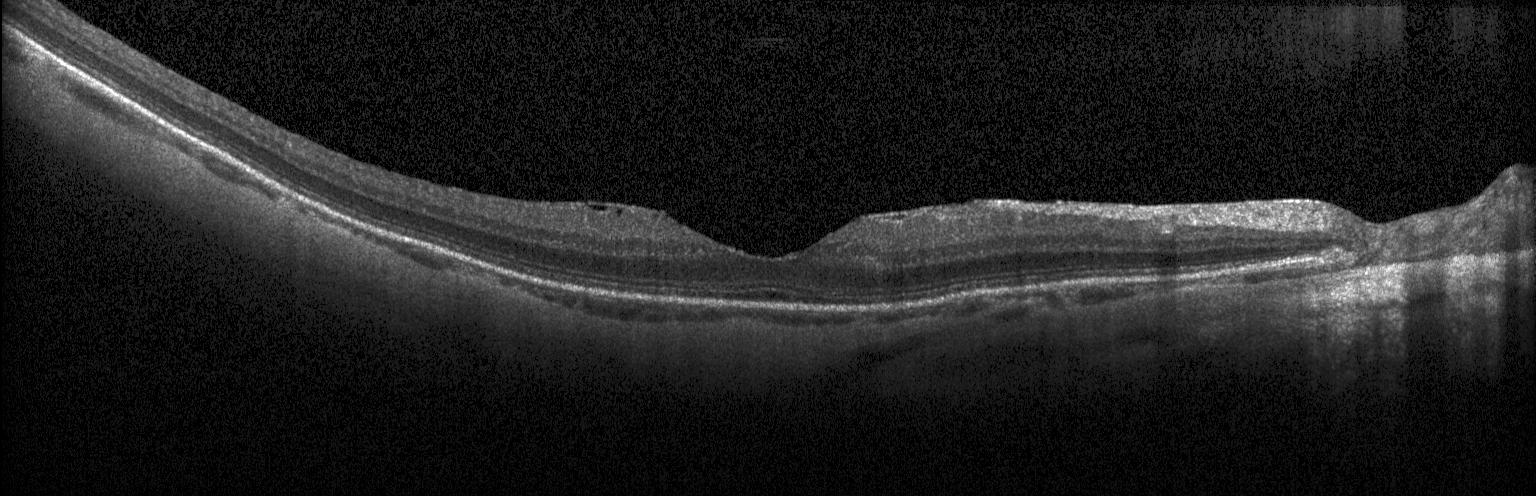 Optical coherence tomography B-scan · Heidelberg Spectralis · through the macula · spectral-domain optical coherence tomography
Diagnosis: no evidence of choroidal neovascularization, diabetic macular edema, or drusen.